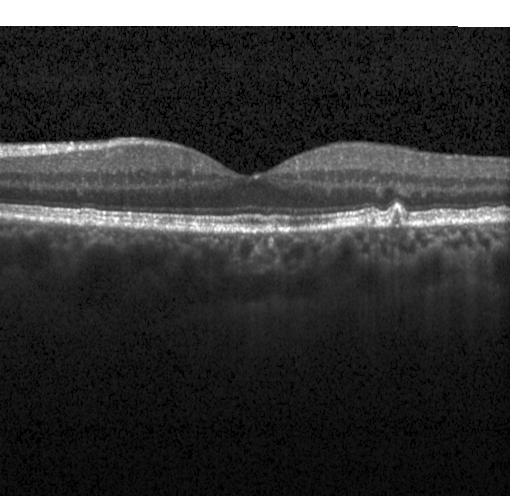
Fovea-centered · optical coherence tomography B-scan · instrument: Heidelberg Spectralis · spectral-domain optical coherence tomography
Finding: multiple drusen.